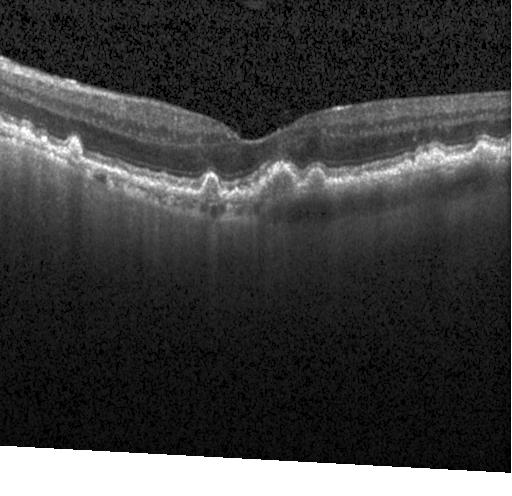
Retinal OCT cross-section; fovea-centered. OCT finding: sub-RPE drusenoid deposits.